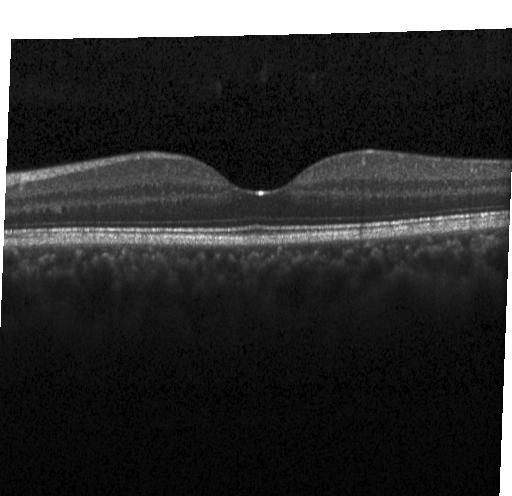
Diagnosis: no choroidal neovascularization, diabetic macular edema, or drusen.